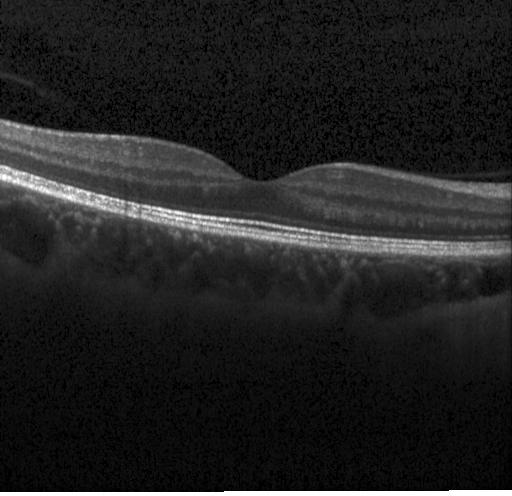 Through the macula, retinal OCT B-scan, Heidelberg Spectralis OCT system
Finding: no evidence of CNV, DME, or drusen.